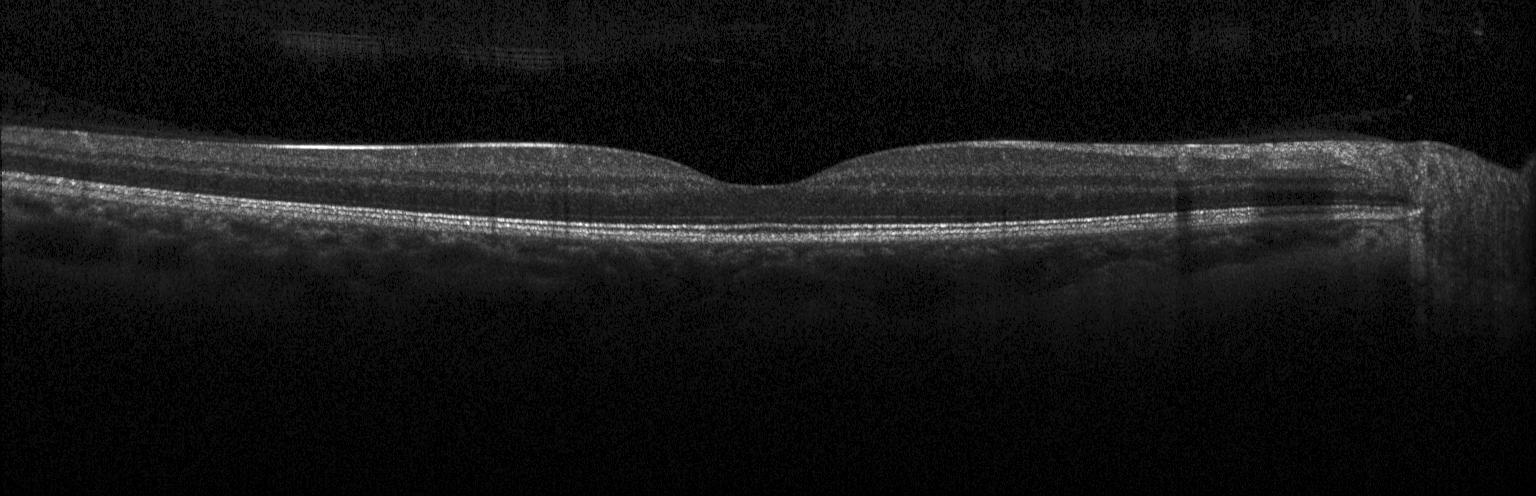 Spectral-domain OCT B-scan: no evidence of CNV, DME, or drusen.